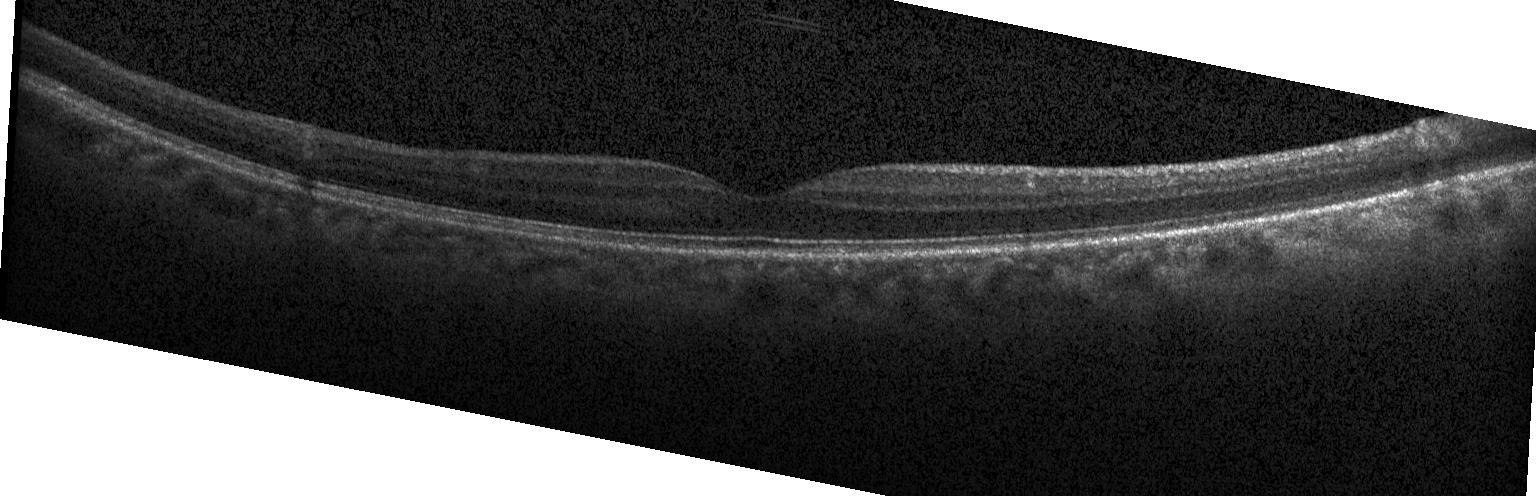 No CNV, no DME, and no drusen.